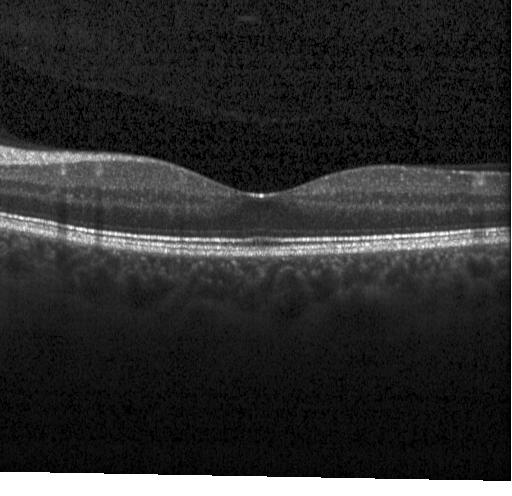

OCT B-scan. No choroidal neovascularization, diabetic macular edema, or drusen.